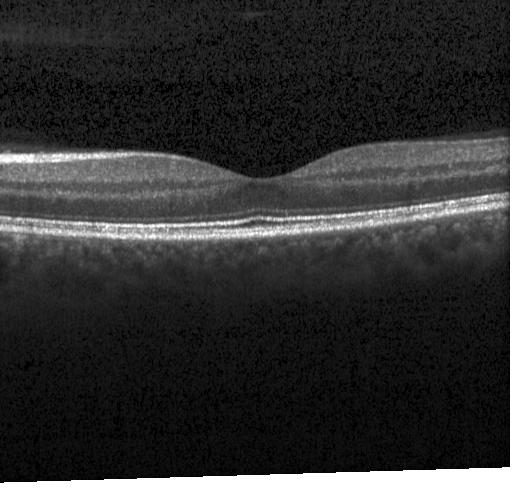

Optical coherence tomography scan
Diagnosis: neither choroidal neovascularization, diabetic macular edema, nor drusen.